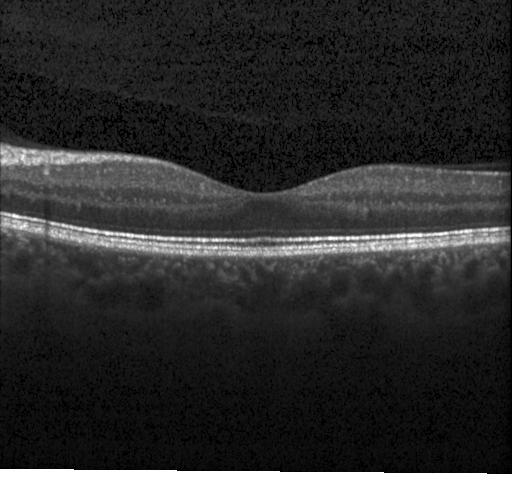 Heidelberg Spectralis, spectral-domain optical coherence tomography, OCT line scan — Diagnosis: neither choroidal neovascularization, diabetic macular edema, nor drusen.